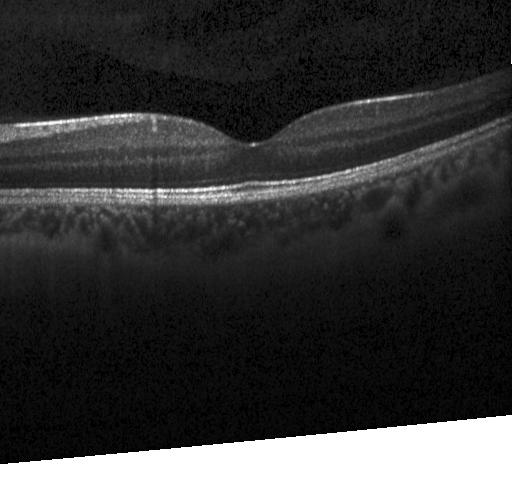
Finding: no choroidal neovascularization, no diabetic macular edema, and no drusen.